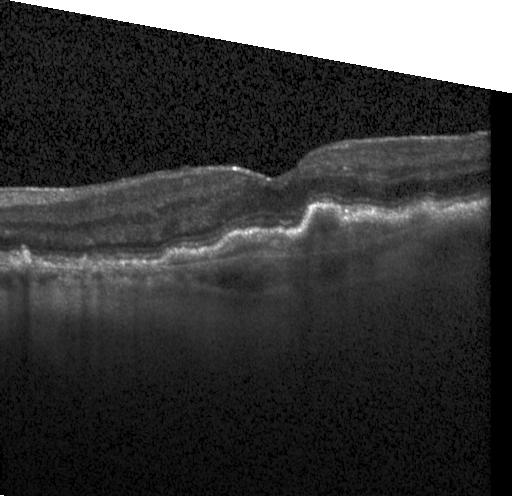
Retinal OCT B-scan.
Assessment: a choroidal neovascular membrane.